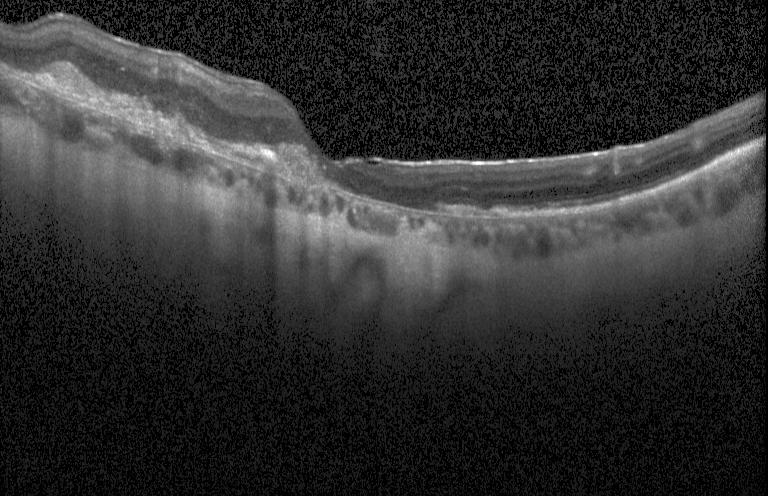

Heidelberg Spectralis OCT system. Optical coherence tomography B-scan.
Macular OCT: a choroidal neovascular membrane.